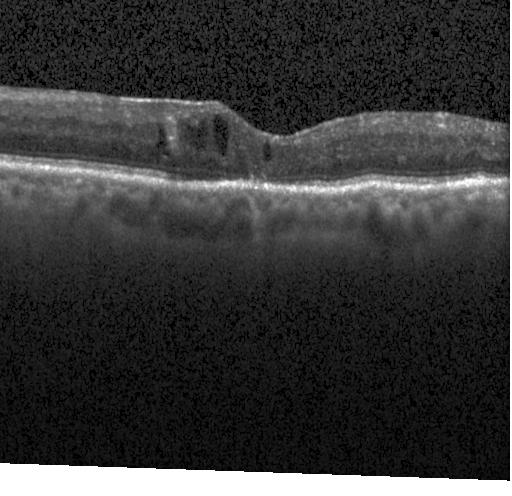 OCT line scan · spectral-domain OCT · horizontal scan through the fovea
Diagnosis: DME.